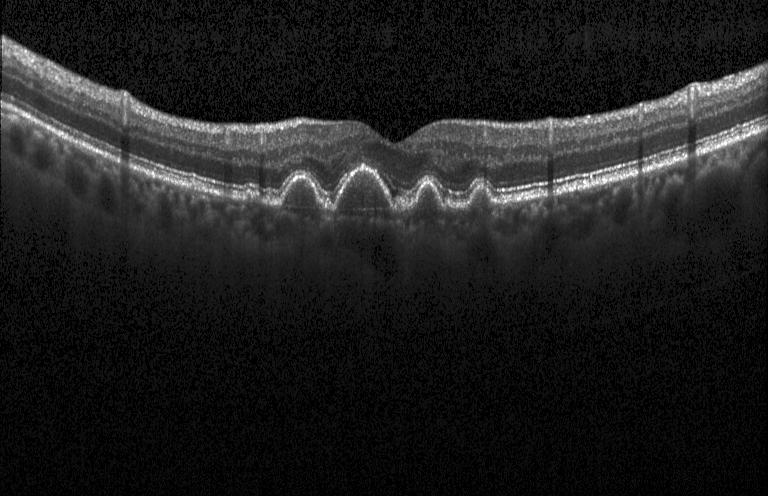

Finding: drusen.